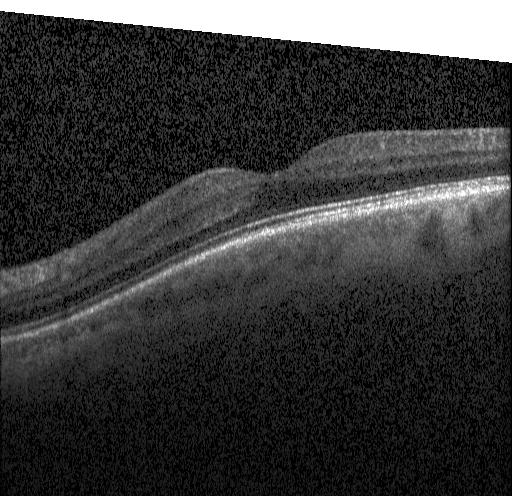
Spectral-domain OCT B-scan: no choroidal neovascularization, diabetic macular edema, or drusen.